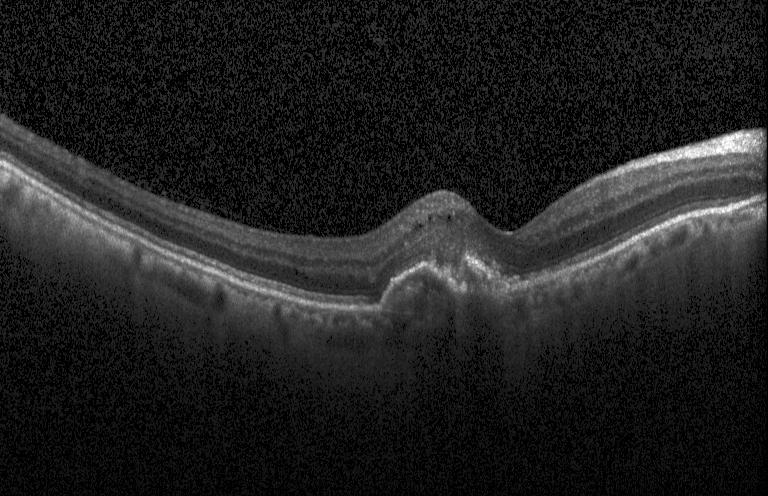
OCT finding: CNV.